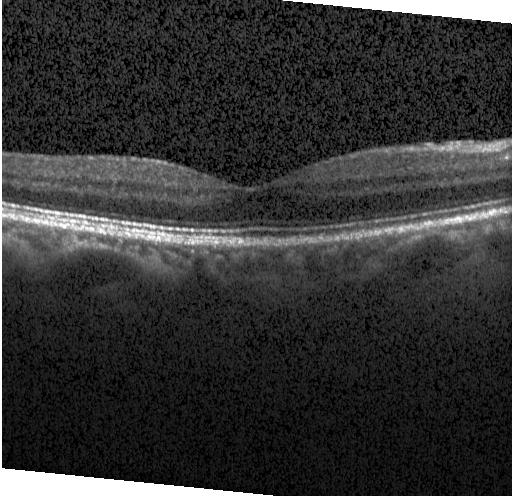

Diagnosis: no choroidal neovascularization, no diabetic macular edema, and no drusen.